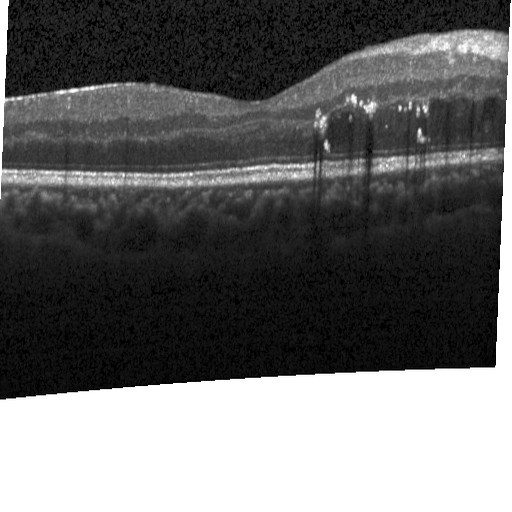
Diagnosis: diabetic macular edema.